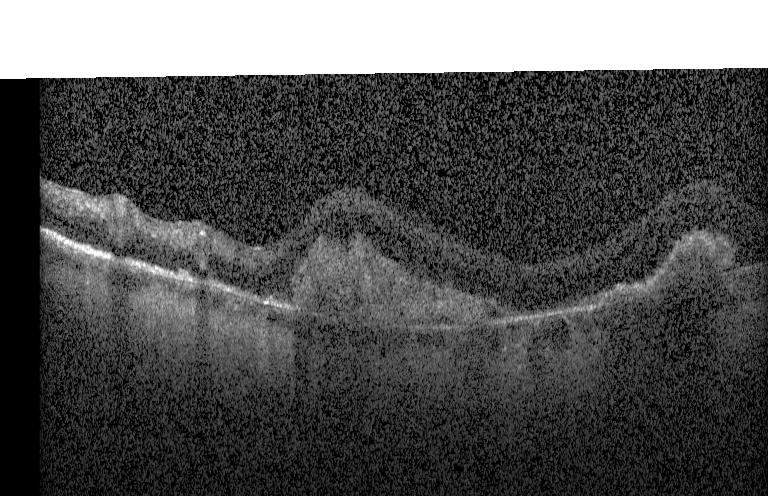
Heidelberg Spectralis OCT system; OCT line scan; spectral-domain OCT. CNV.